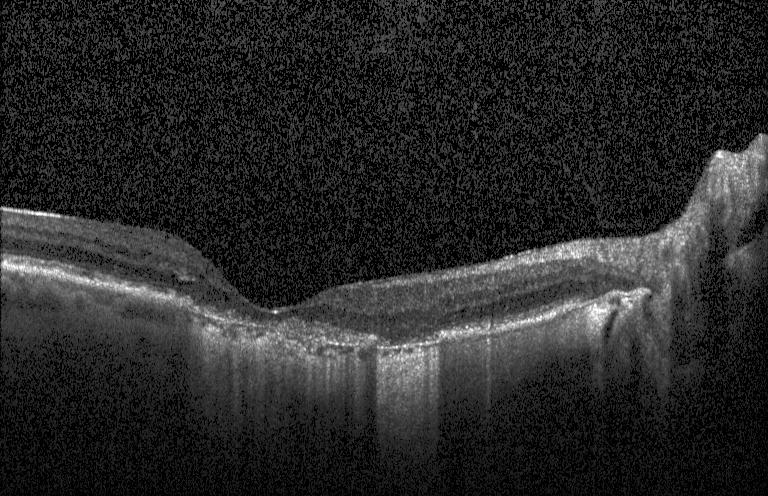 Diagnosis: a choroidal neovascular membrane.